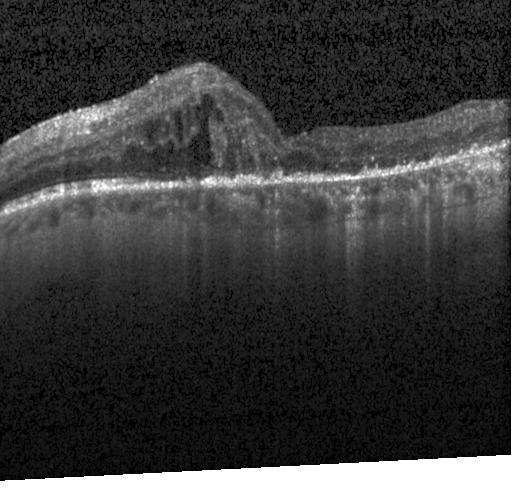

This B-scan demonstrates DME.